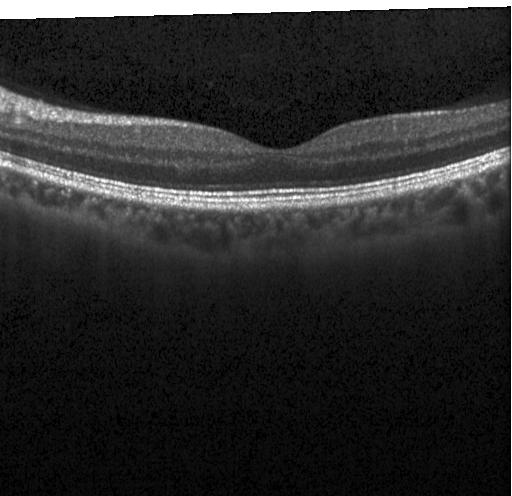

Centered on the fovea. Instrument: Heidelberg Spectralis. Spectral-domain OCT. Retinal OCT B-scan — Finding: no choroidal neovascularization, diabetic macular edema, or drusen.